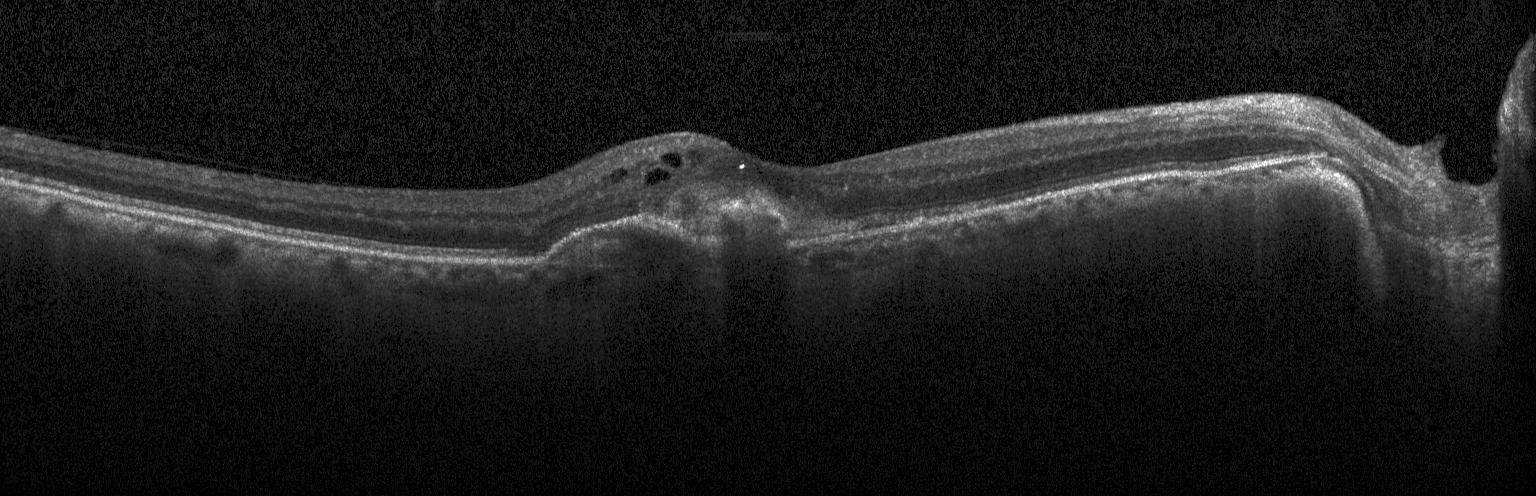

OCT line scan; spectral-domain optical coherence tomography; centered on the fovea
Impression: choroidal neovascularization.